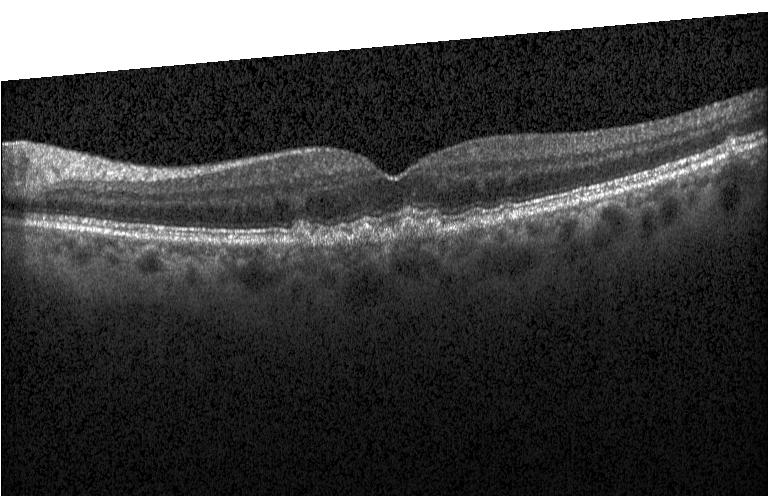

Retinal OCT cross-section showing sub-RPE drusenoid deposits.